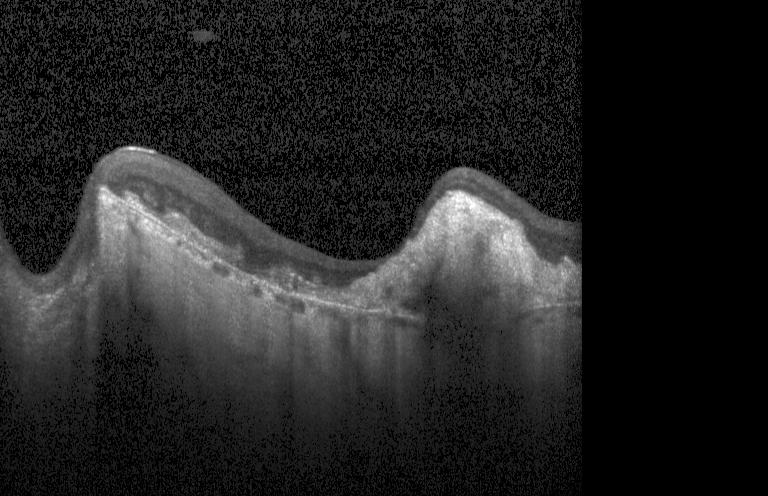

Dx: choroidal neovascularization (CNV).